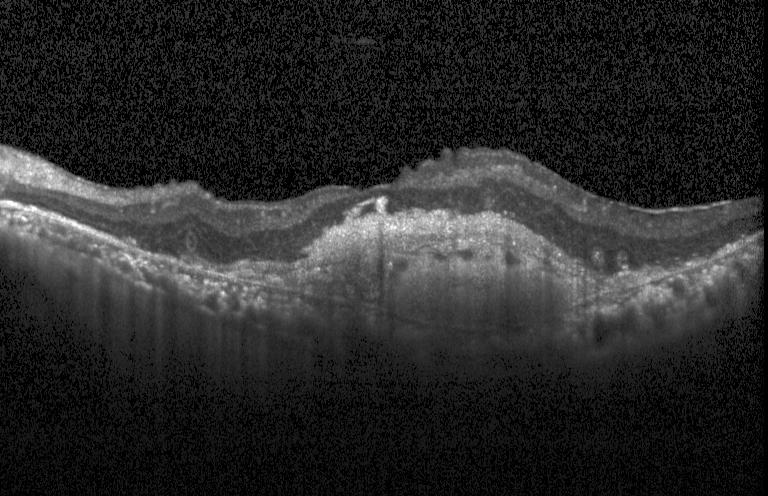

Optical coherence tomography B-scan.
A choroidal neovascular membrane.